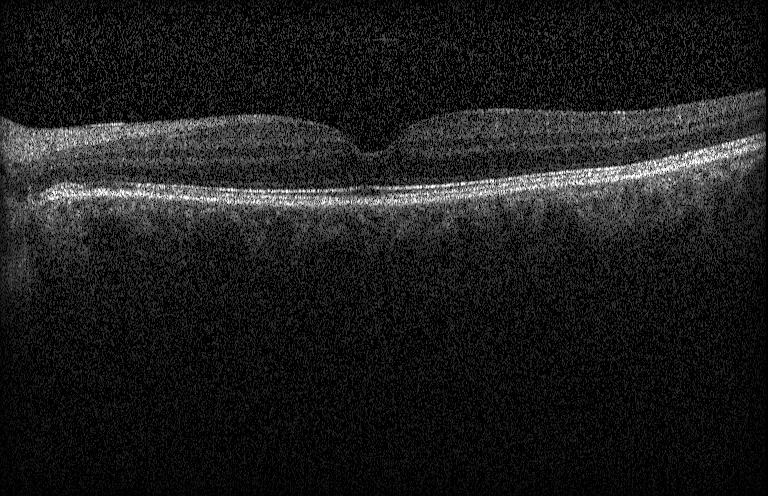 Spectral-domain OCT · through the macula · acquired on a Heidelberg Spectralis · optical coherence tomography B-scan
Impression: no choroidal neovascularization, diabetic macular edema, or drusen.